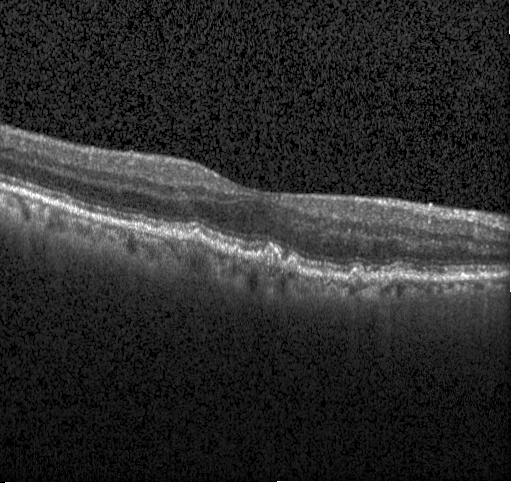 Optical coherence tomography scan; SD-OCT. OCT finding: multiple drusen.